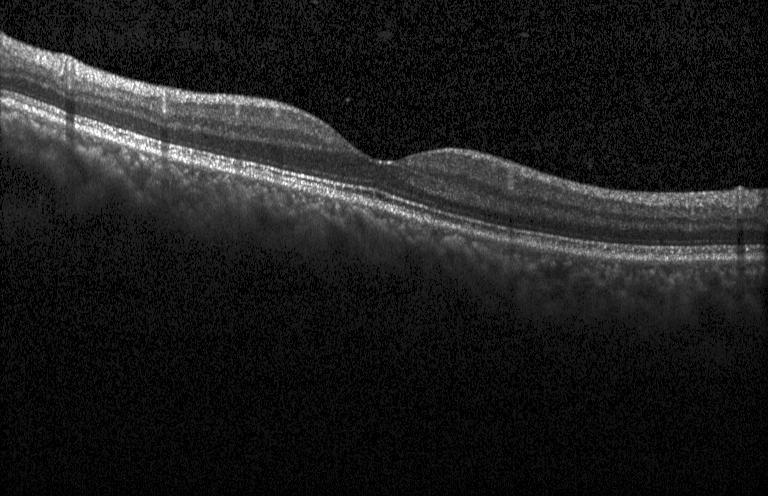 Optical coherence tomography B-scan
This B-scan demonstrates neither CNV, DME, nor drusen.